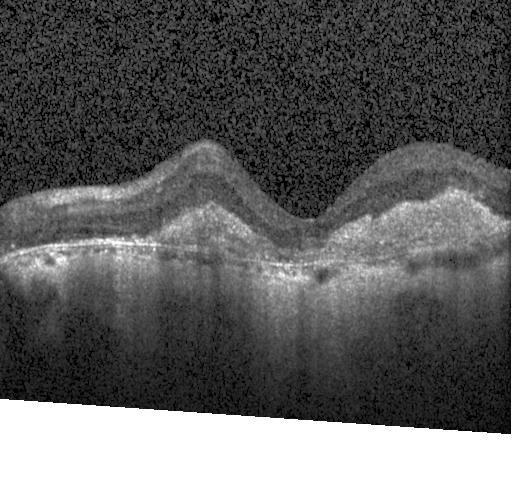
Retinal OCT B-scan; spectral-domain optical coherence tomography.
Impression: a choroidal neovascular membrane.